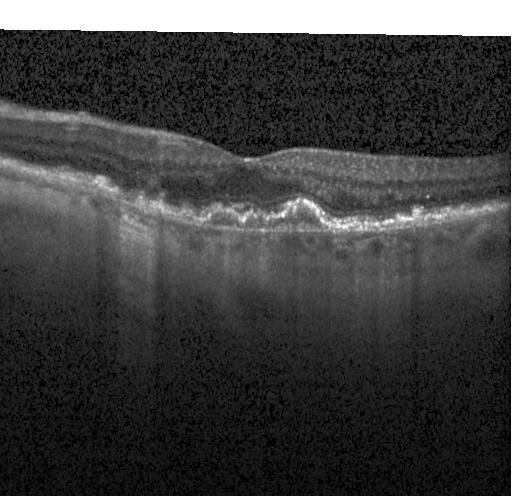

Macular OCT demonstrating a choroidal neovascular membrane.